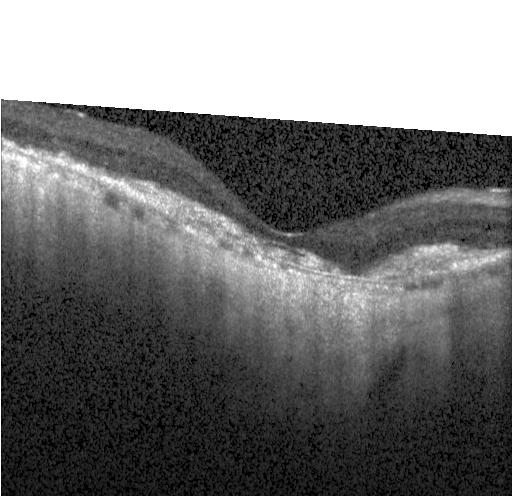
OCT B-scan, spectral-domain OCT, horizontal scan through the fovea — CNV.